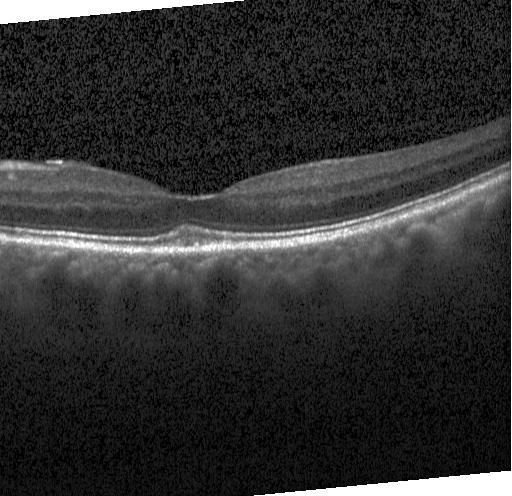 Finding: no evidence of CNV, DME, or drusen.